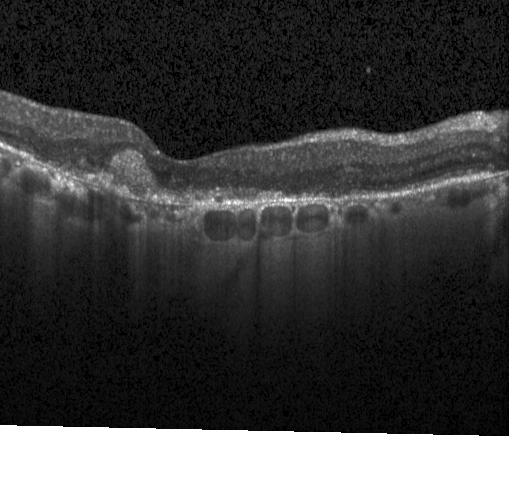

Optical coherence tomography B-scan; fovea-centered. Impression: CNV.